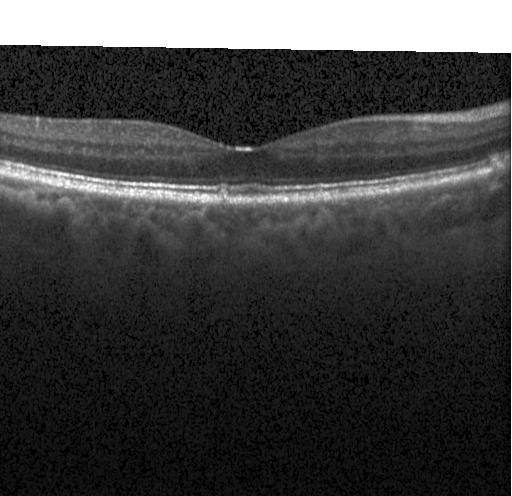

Finding: no evidence of choroidal neovascularization, diabetic macular edema, or drusen.